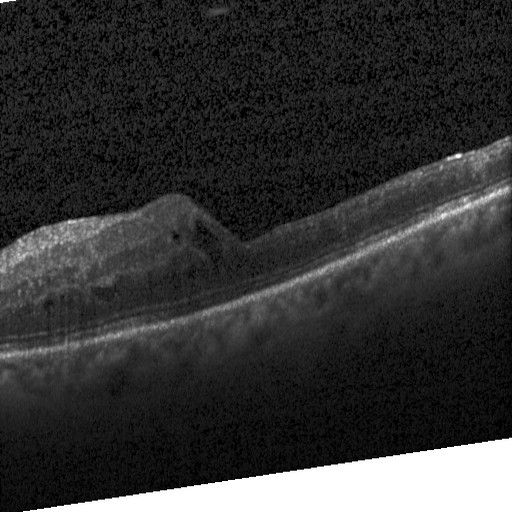 OCT B-scan. Spectral-domain OCT. Instrument: Heidelberg Spectralis. Through the macula
This B-scan demonstrates diabetic macular edema (DME).